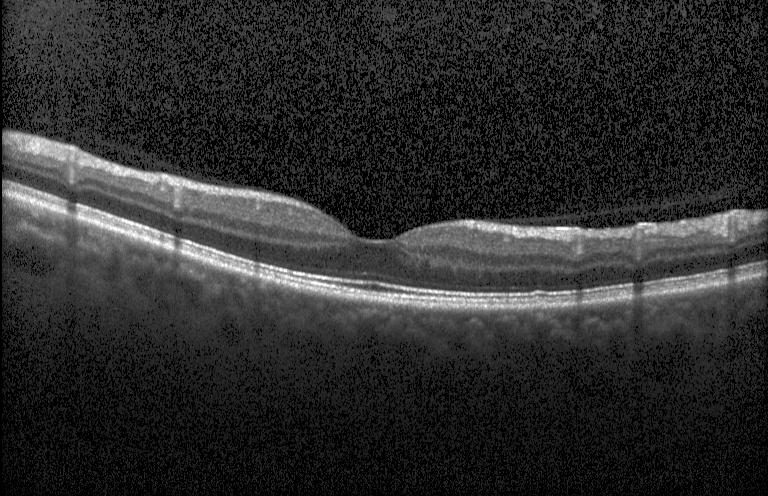
Spectral-domain OCT B-scan: no CNV, no DME, and no drusen.